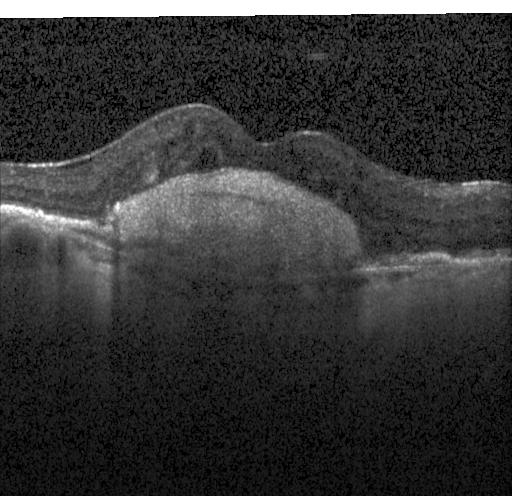

Retinal OCT B-scan.
Impression: choroidal neovascularization.